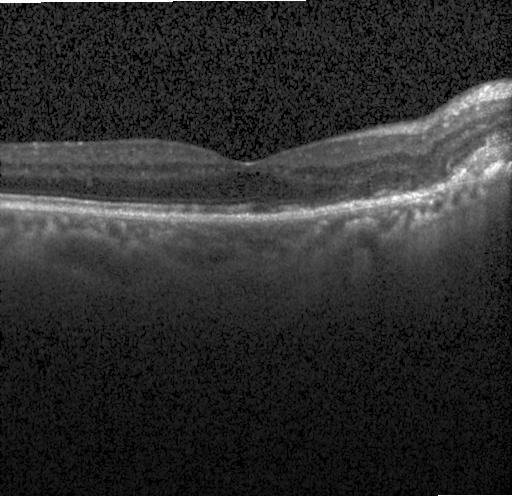
Spectral-domain optical coherence tomography; retinal OCT B-scan; macular scan. Diagnosis: choroidal neovascularization (CNV).